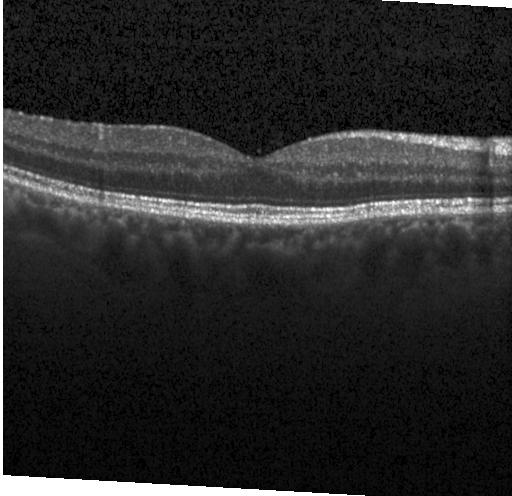 Macular OCT: neither choroidal neovascularization, diabetic macular edema, nor drusen.